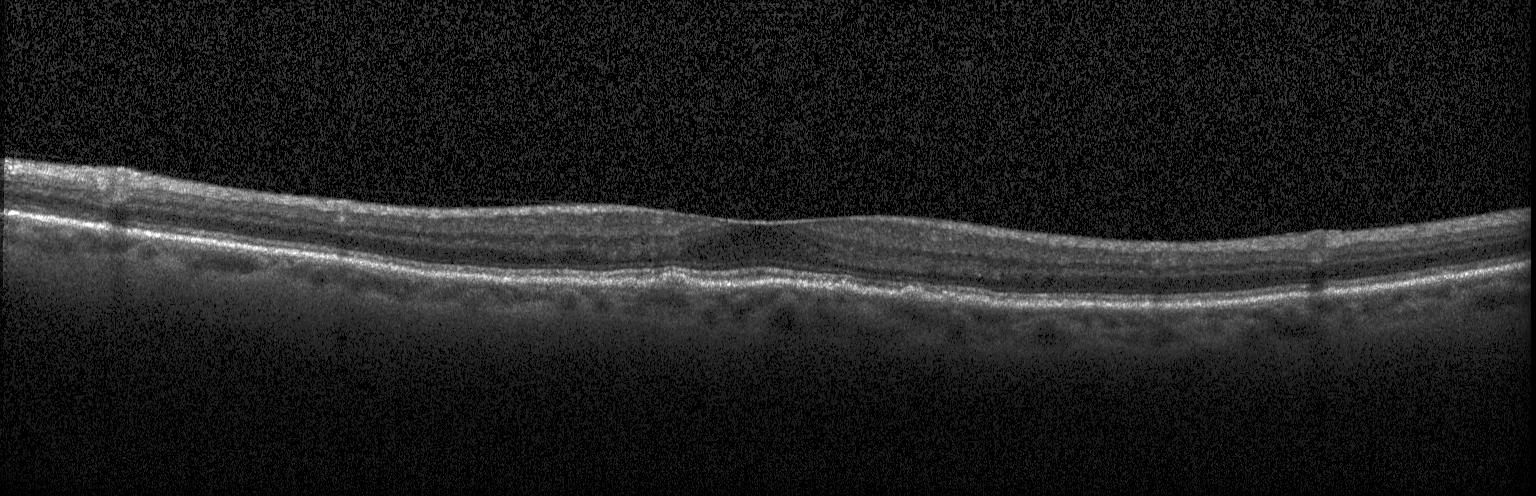
Acquired on a Heidelberg Spectralis, retinal OCT cross-section — Drusen.